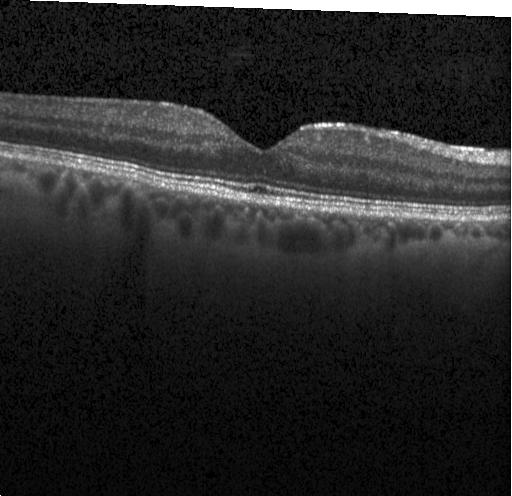 Fovea-centered. Instrument: Heidelberg Spectralis. Retinal OCT B-scan. Spectral-domain optical coherence tomography
Diagnosis: neither choroidal neovascularization, diabetic macular edema, nor drusen.